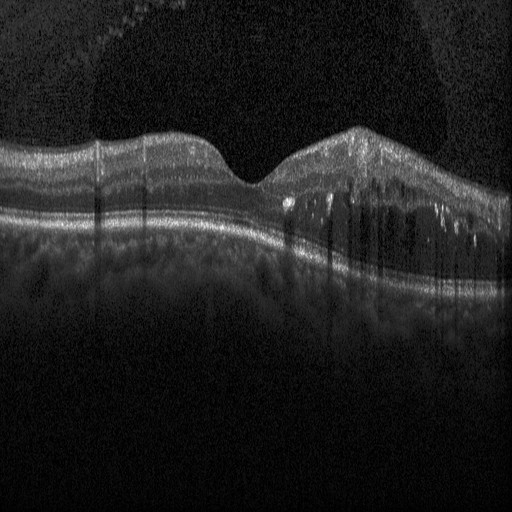 Retinal OCT B-scan · spectral-domain OCT.
Assessment: diabetic macular edema.